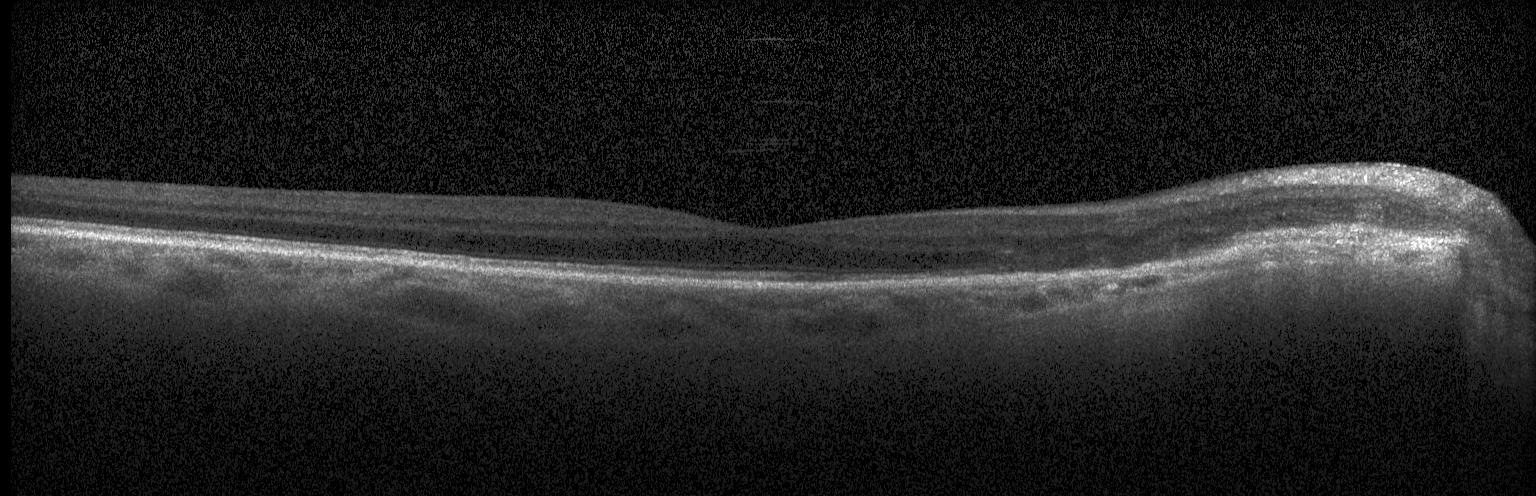
Fovea-centered; retinal OCT cross-section; SD-OCT — Diagnosis: a choroidal neovascular membrane.